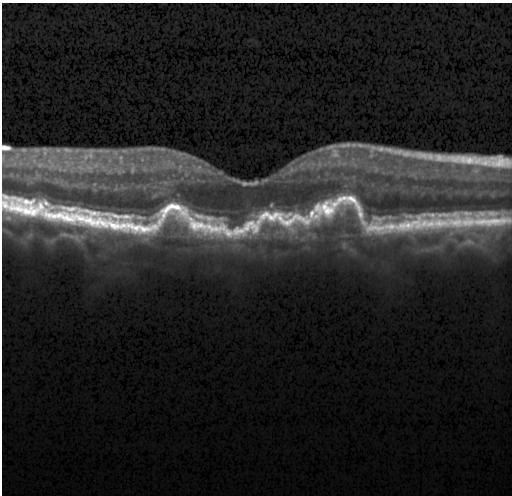
Dx: drusen.